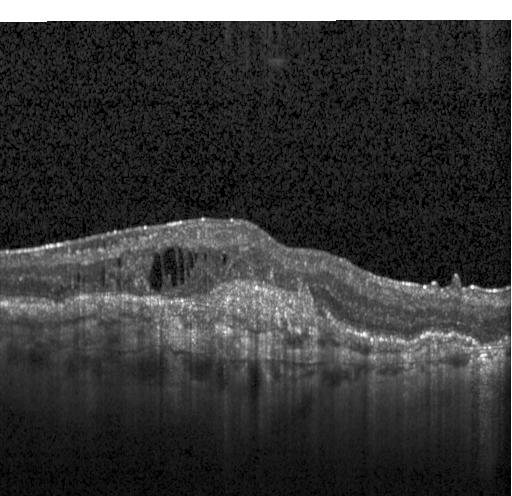

Diagnosis: choroidal neovascularization.